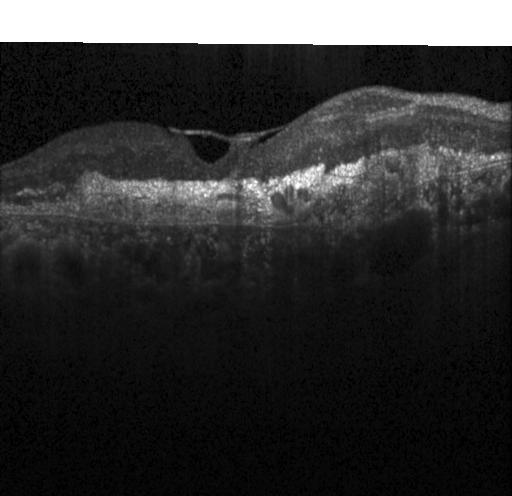

Heidelberg Spectralis, retinal OCT cross-section.
Impression: CNV.